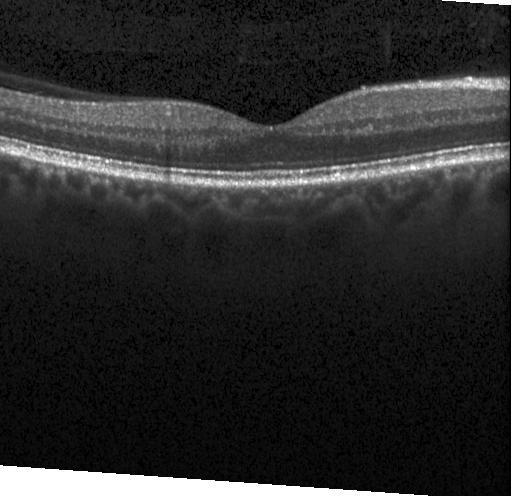
OCT scan showing neither choroidal neovascularization, diabetic macular edema, nor drusen.